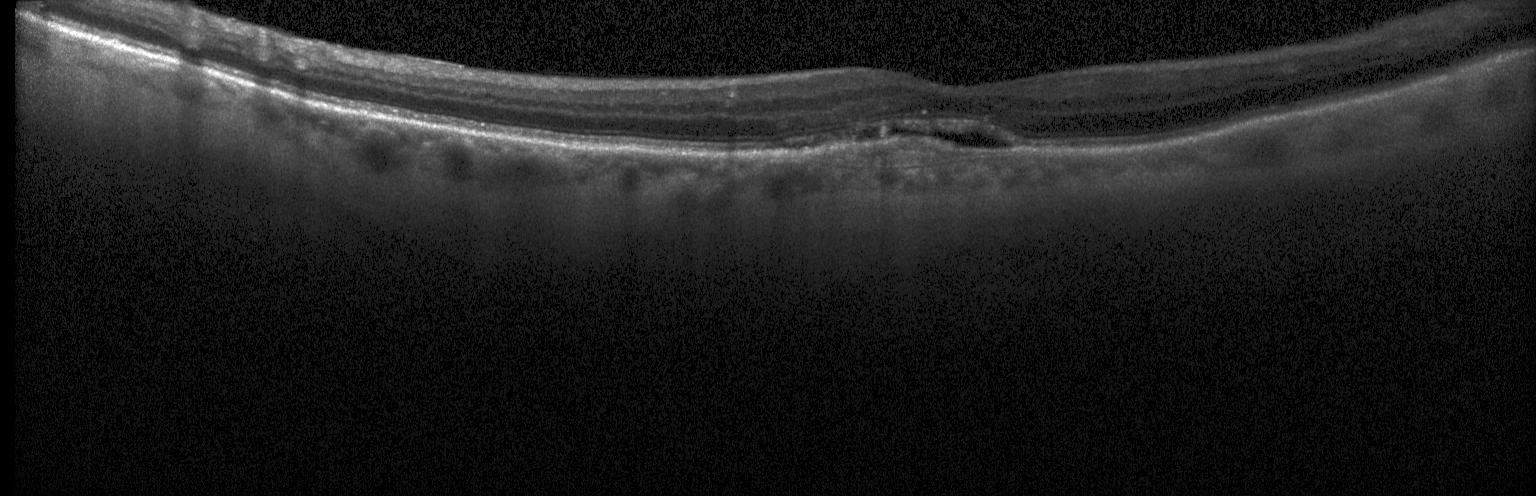
Choroidal neovascularization.